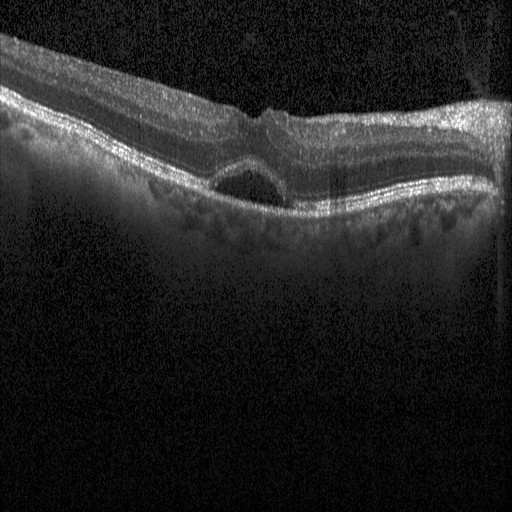
Centered on the fovea; retinal OCT cross-section
Impression: diabetic macular edema.